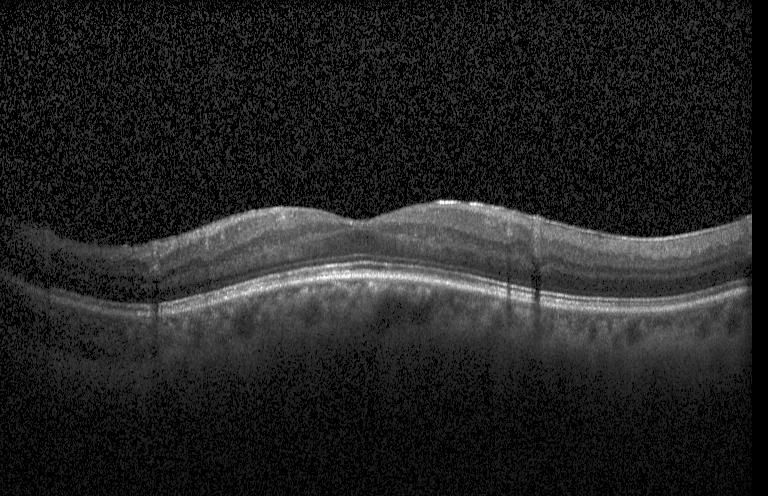 OCT B-scan · spectral-domain OCT · centered on the fovea · instrument: Heidelberg Spectralis.
Impression: no CNV, no DME, and no drusen.